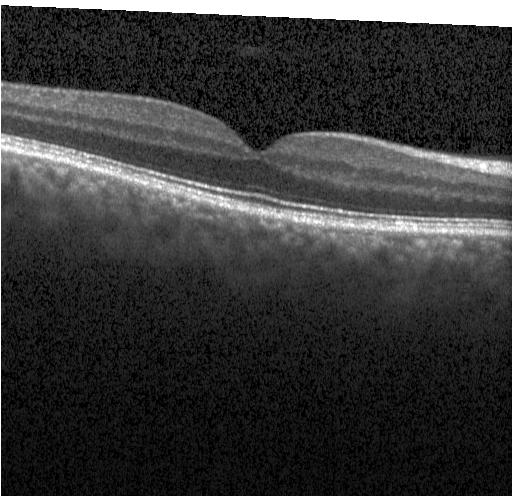

Heidelberg Spectralis OCT system; retinal OCT cross-section; through the macula — Assessment: no choroidal neovascularization, no diabetic macular edema, and no drusen.